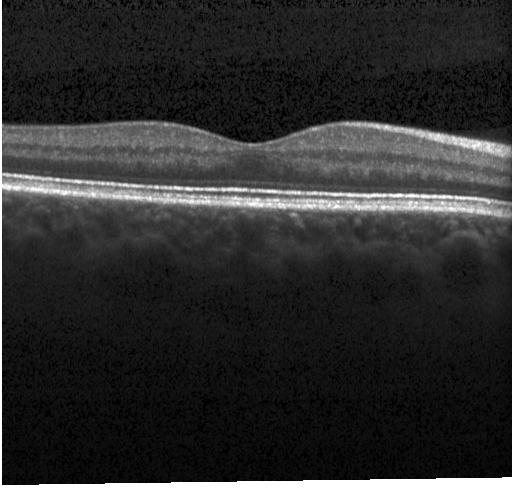
Spectral-domain OCT B-scan: no choroidal neovascularization, diabetic macular edema, or drusen.